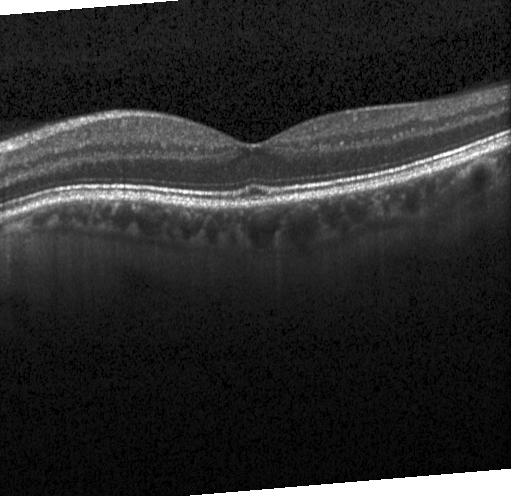

Spectral-domain optical coherence tomography; optical coherence tomography scan — Finding: neither choroidal neovascularization, diabetic macular edema, nor drusen.